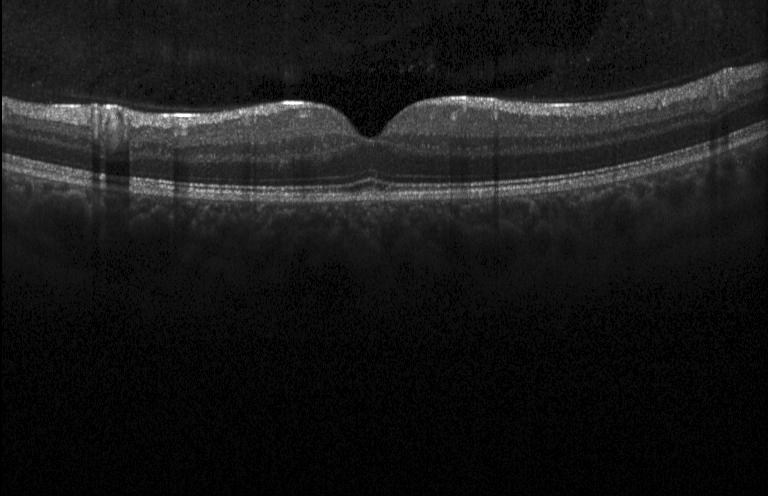

Finding: no evidence of choroidal neovascularization, diabetic macular edema, or drusen.